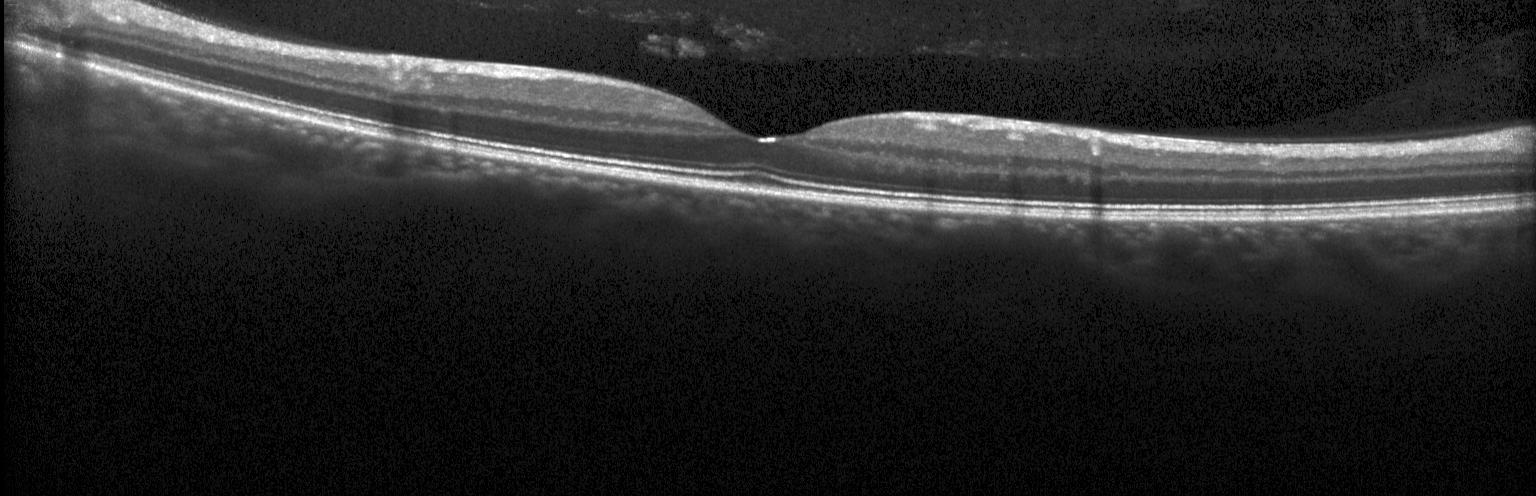 Retinal OCT B-scan
Diagnosis: no evidence of CNV, DME, or drusen.